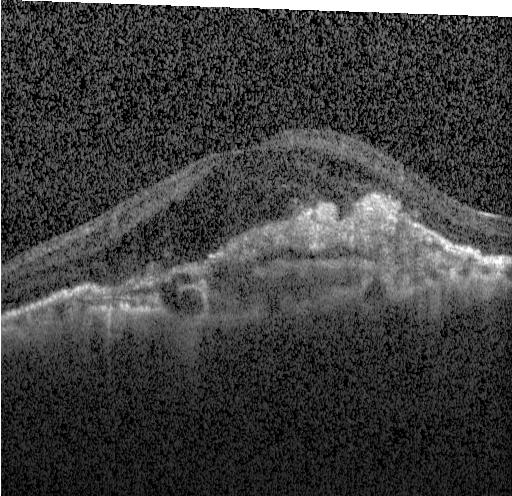

Finding: choroidal neovascularization (CNV).